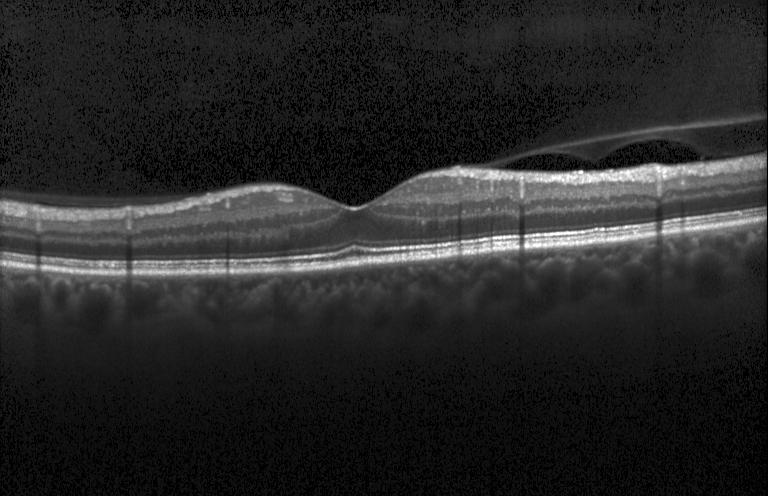

Macular scan; Heidelberg Spectralis OCT system; optical coherence tomography B-scan; SD-OCT.
Impression: neither choroidal neovascularization, diabetic macular edema, nor drusen.